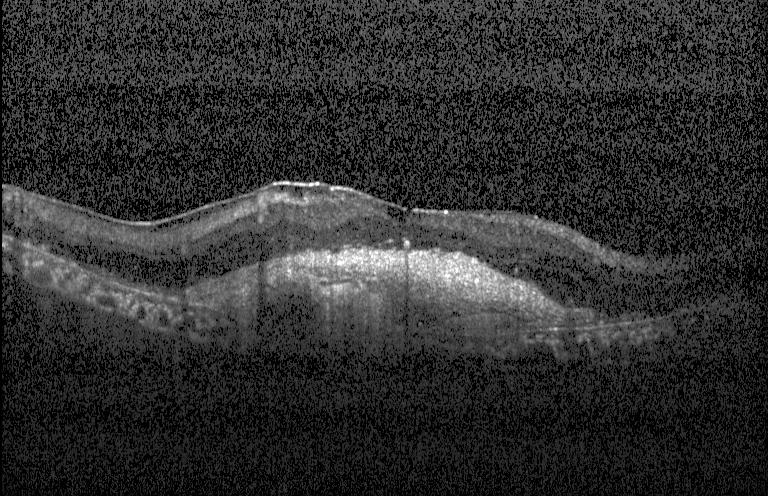
Fovea-centered · optical coherence tomography scan · SD-OCT. Diagnosis: choroidal neovascularization.